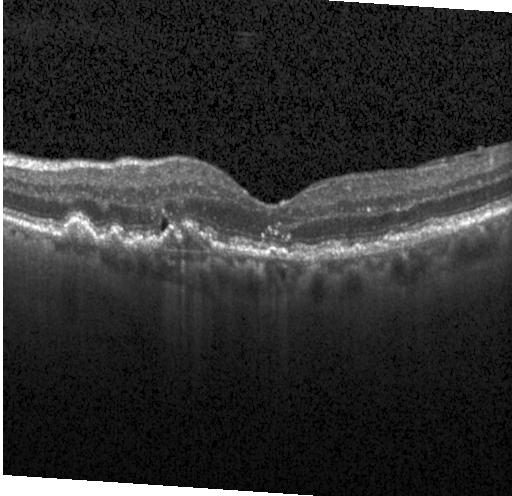

Macular OCT: a choroidal neovascular membrane.